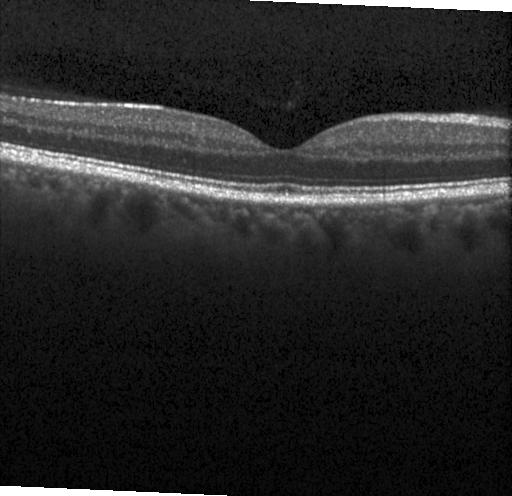

Retinal OCT B-scan, SD-OCT, instrument: Heidelberg Spectralis — Finding: no CNV, no DME, and no drusen.